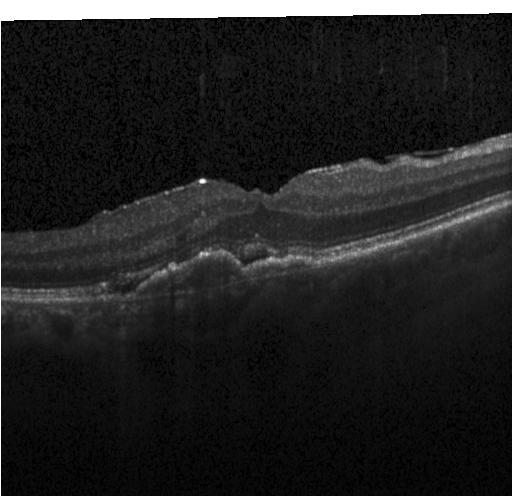 The scan shows choroidal neovascularization (CNV).